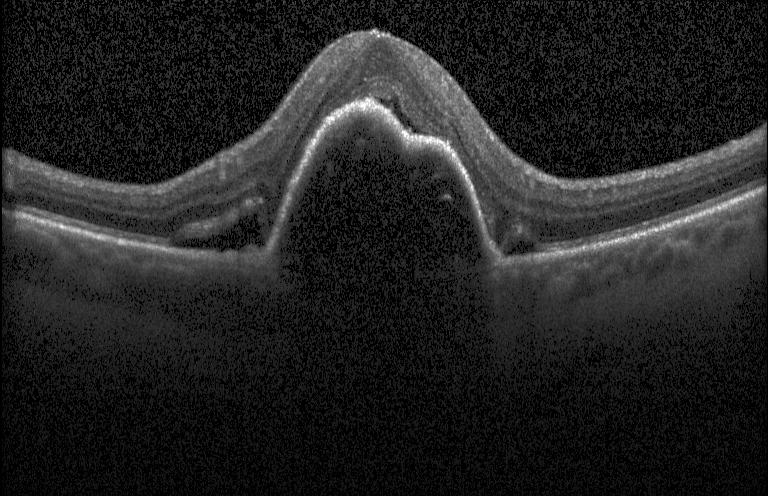
Spectral-domain optical coherence tomography · macular scan · OCT line scan · Heidelberg Spectralis OCT system. The scan shows a choroidal neovascular membrane.